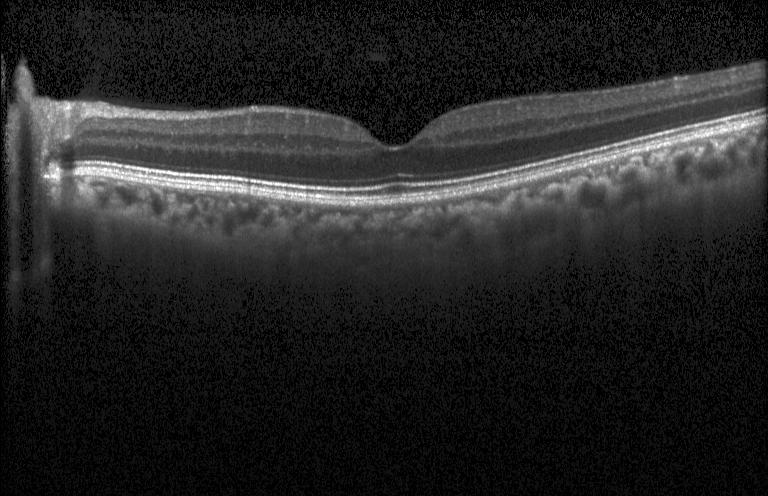
Spectral-domain optical coherence tomography. Retinal OCT cross-section. Diagnosis: no choroidal neovascularization, no diabetic macular edema, and no drusen.